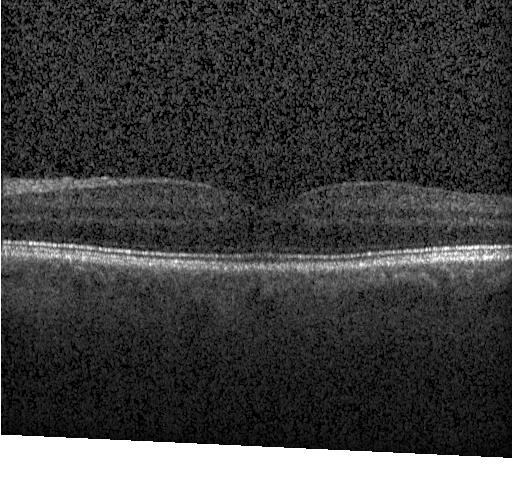

No CNV, DME, or drusen.